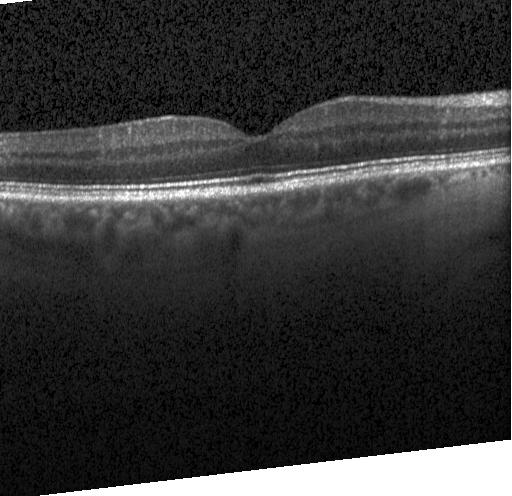 OCT line scan · centered on the fovea · Heidelberg Spectralis · spectral-domain optical coherence tomography — Assessment: no choroidal neovascularization, no diabetic macular edema, and no drusen.